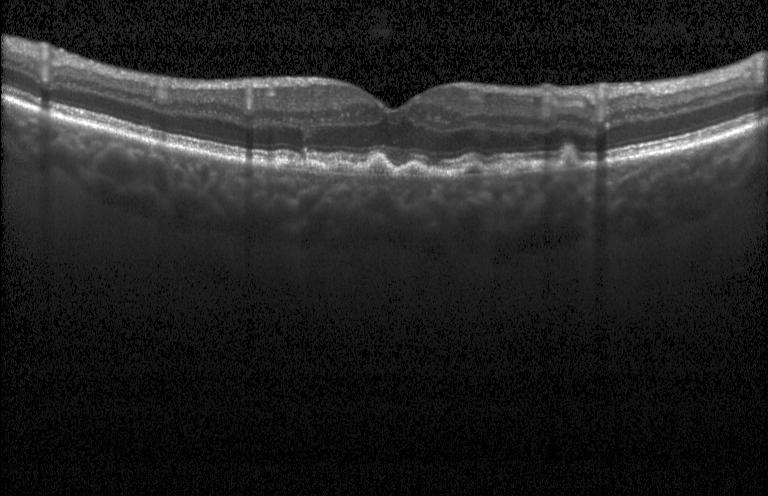
Diagnosis: sub-RPE drusenoid deposits.